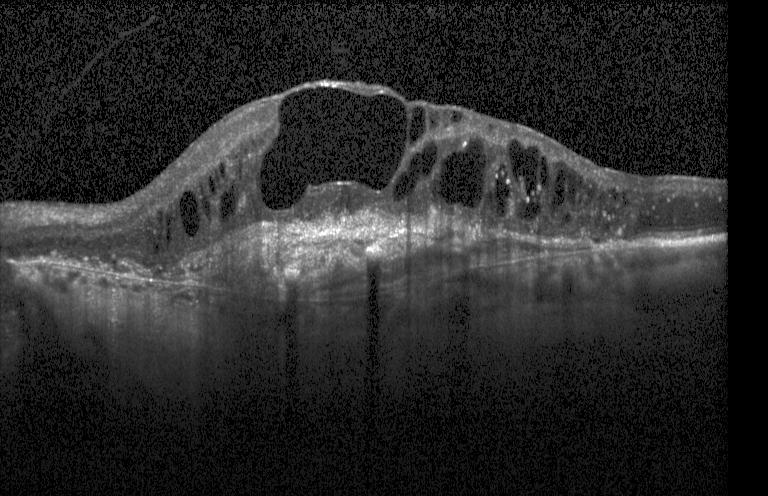

Finding: a choroidal neovascular membrane.